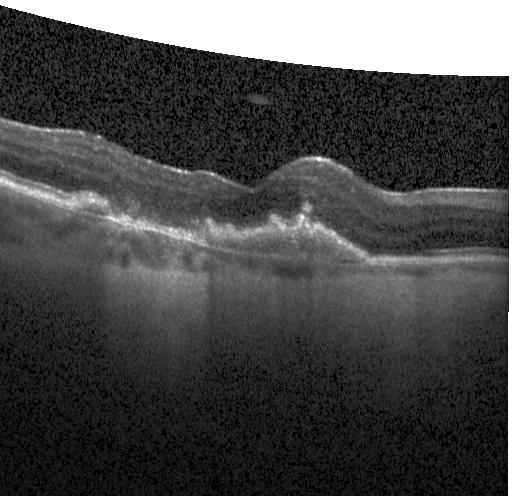
Optical coherence tomography B-scan; SD-OCT; instrument: Heidelberg Spectralis — Diagnosis: choroidal neovascularization (CNV).